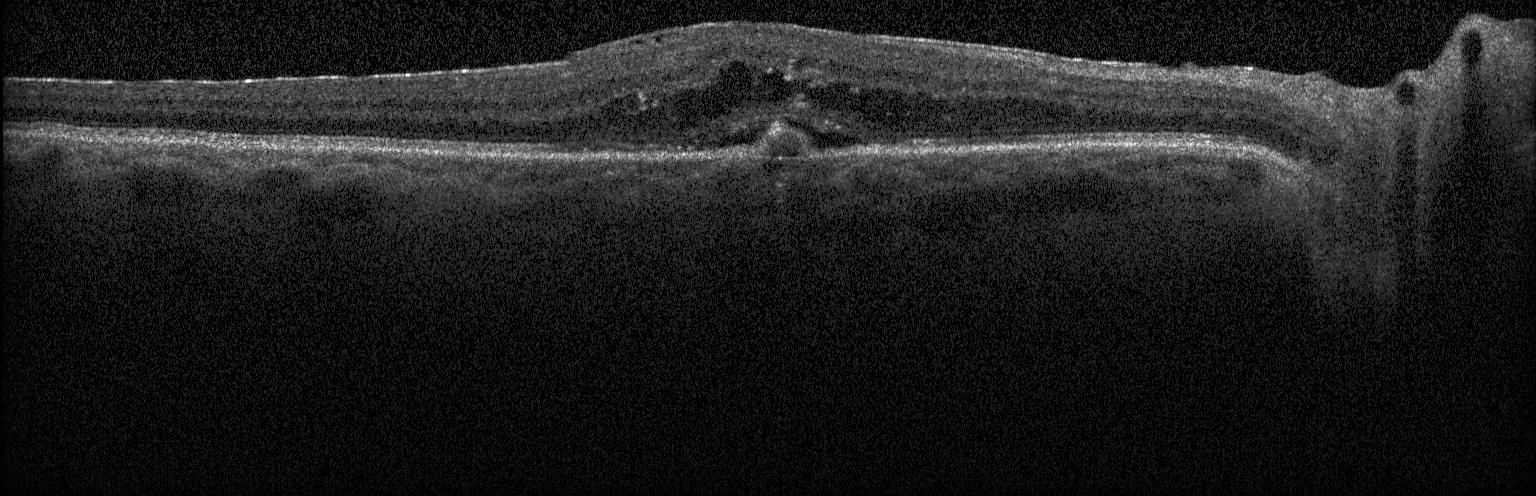

Fovea-centered; SD-OCT; OCT B-scan; Heidelberg Spectralis OCT system.
Diagnosis: CNV.